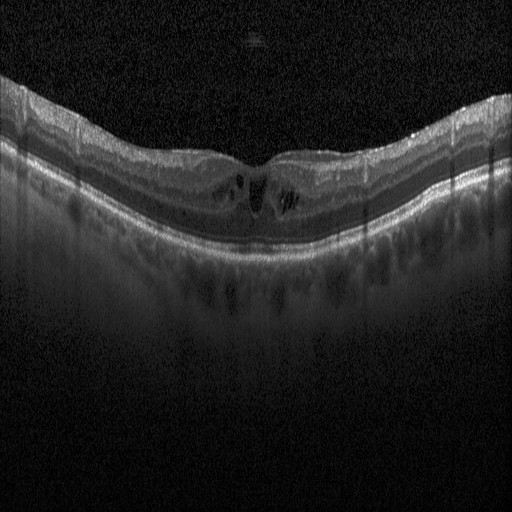 Dx: diabetic macular edema.